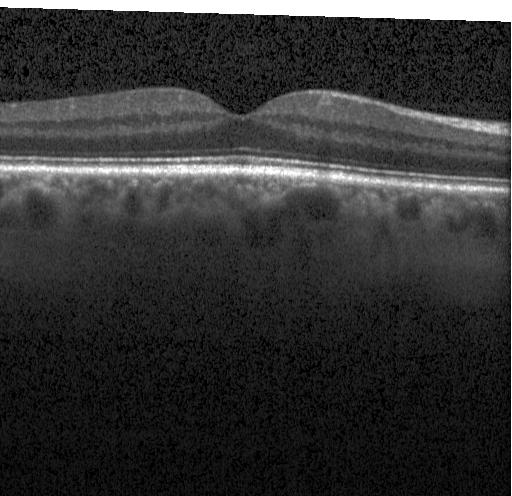
Fovea-centered; optical coherence tomography B-scan; spectral-domain optical coherence tomography; Heidelberg Spectralis OCT system
Diagnosis: no evidence of CNV, DME, or drusen.